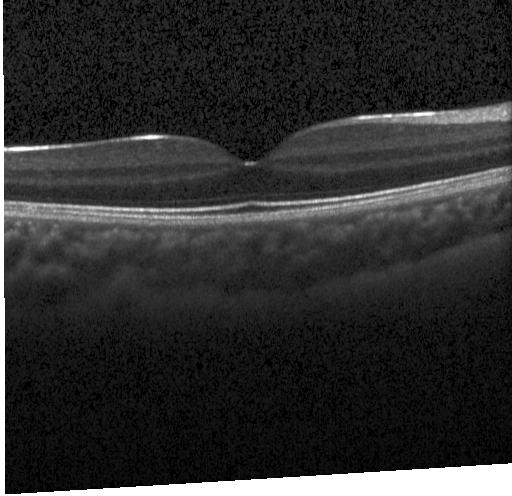 Retinal OCT B-scan. Heidelberg Spectralis.
Assessment: neither CNV, DME, nor drusen.